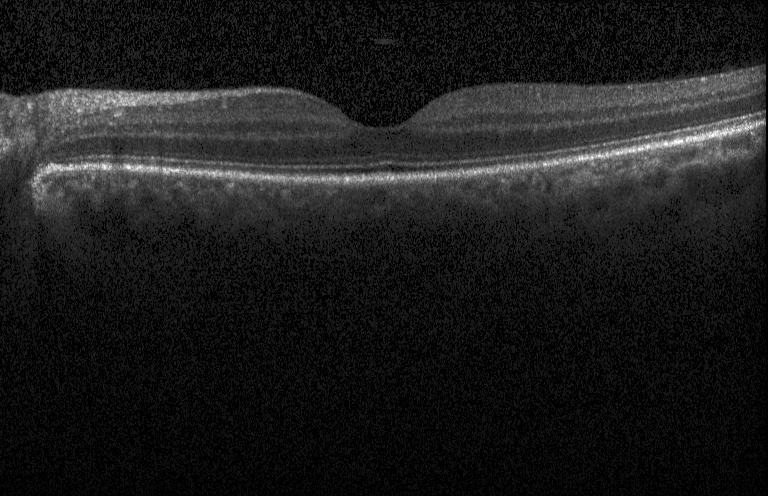
Optical coherence tomography B-scan; centered on the fovea; spectral-domain optical coherence tomography
Finding: no CNV, DME, or drusen.